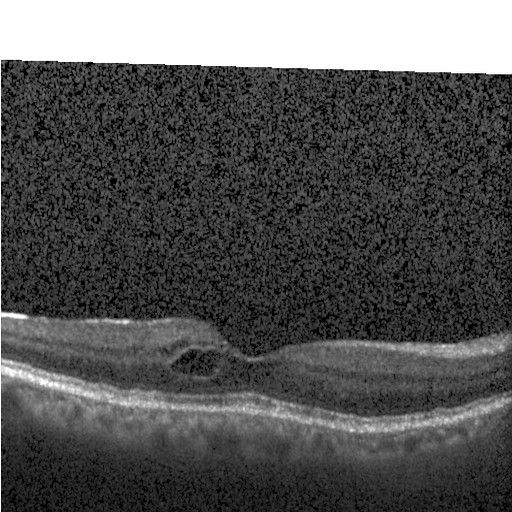
Optical coherence tomography scan · instrument: Heidelberg Spectralis · horizontal scan through the fovea — Diagnosis: DME.